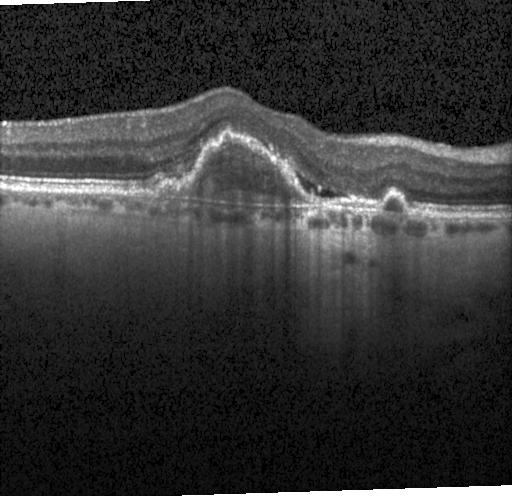

Fovea-centered. Spectral-domain optical coherence tomography. Heidelberg Spectralis. OCT line scan — This B-scan demonstrates a choroidal neovascular membrane.